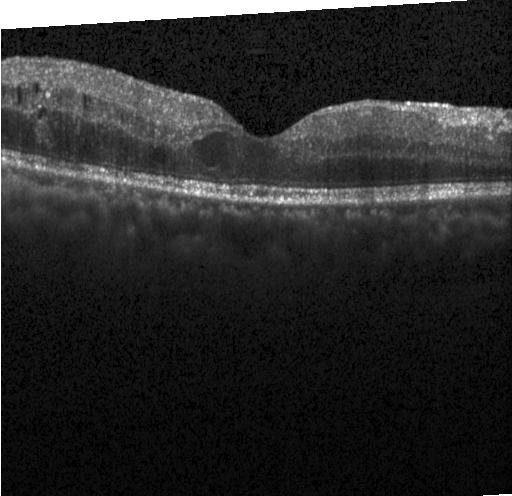

OCT B-scan showing diabetic macular edema (DME).